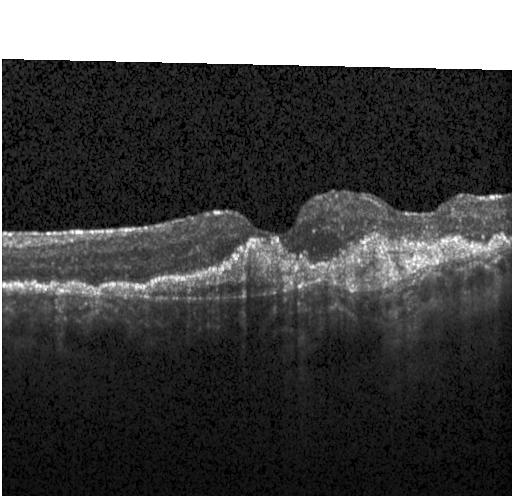
Impression: a choroidal neovascular membrane.